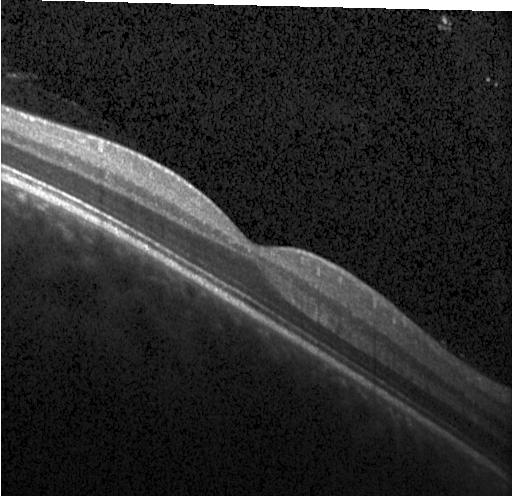

OCT line scan; SD-OCT; macular scan; Heidelberg Spectralis.
No choroidal neovascularization, diabetic macular edema, or drusen.